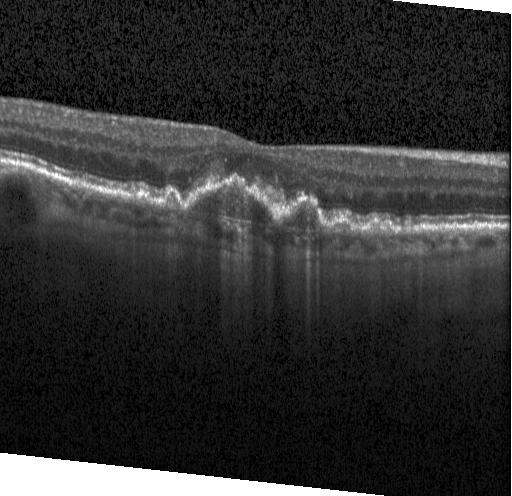

Optical coherence tomography B-scan. Spectral-domain OCT. Heidelberg Spectralis OCT system. Macular scan.
Impression: CNV.